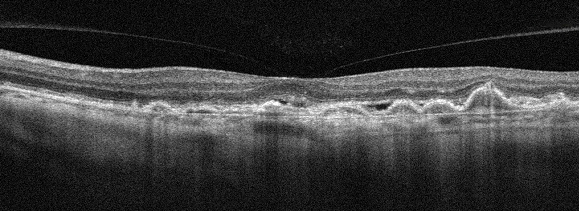
Acquired on an Optovue Avanti RTVue XR; optical coherence tomography scan; left eye — Assessment: age-related macular degeneration.